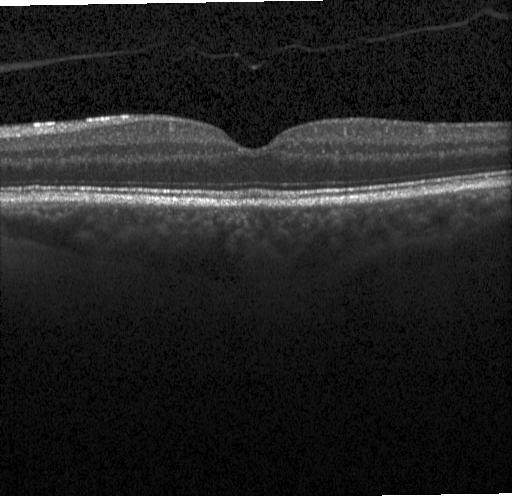

Spectral-domain OCT; retinal OCT B-scan
No CNV, no DME, and no drusen.